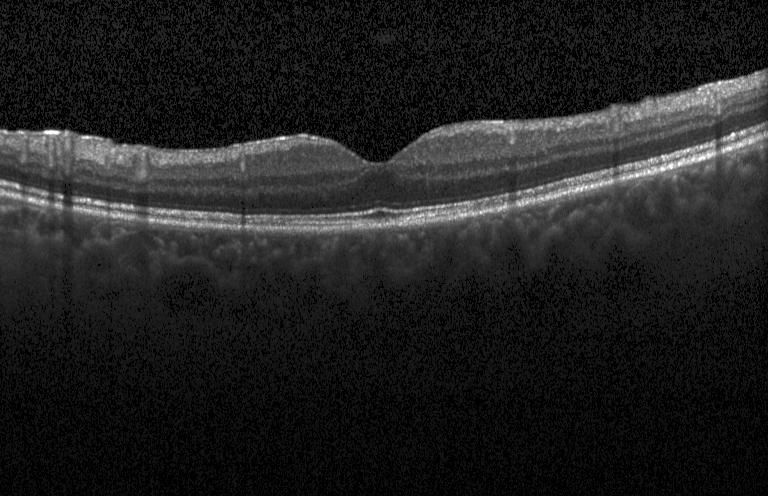 Optical coherence tomography B-scan. Finding: neither CNV, DME, nor drusen.